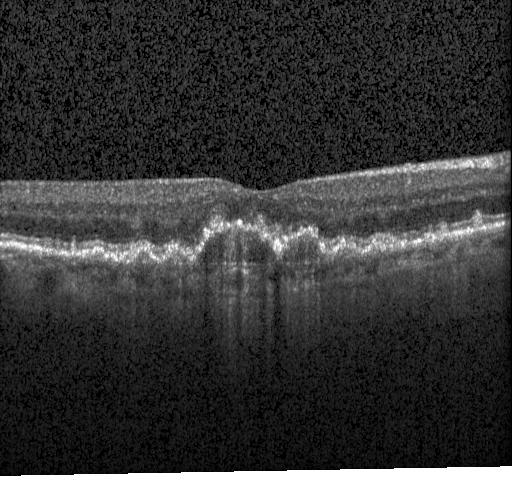 OCT B-scan — CNV.